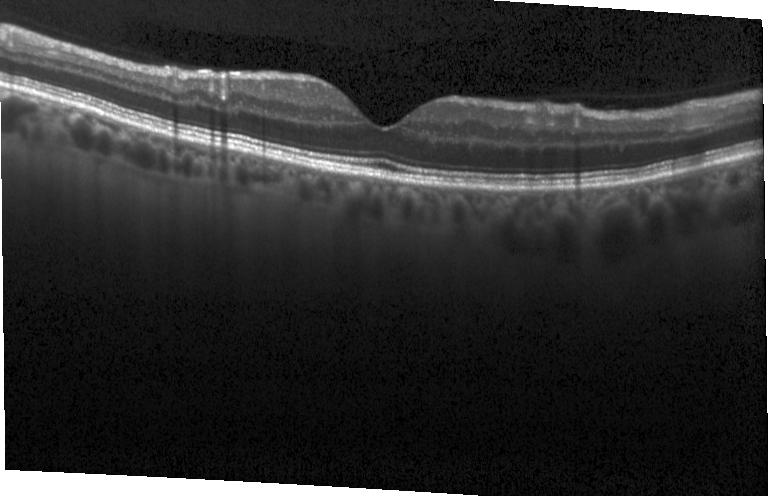
OCT finding: no CNV, DME, or drusen.